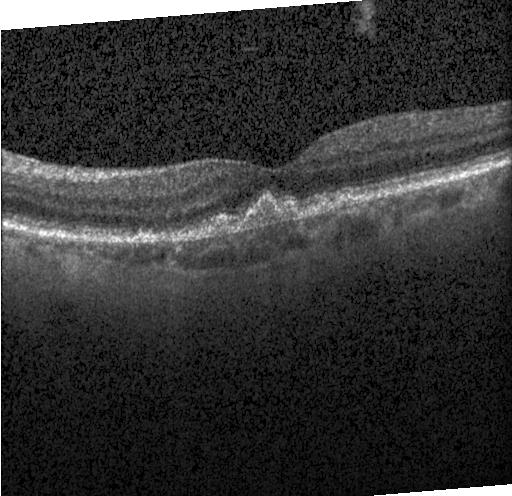
Impression: drusen.